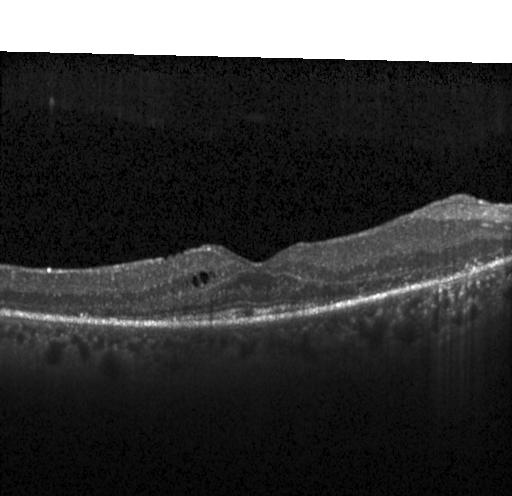
Fovea-centered; optical coherence tomography B-scan — Assessment: diabetic macular edema.